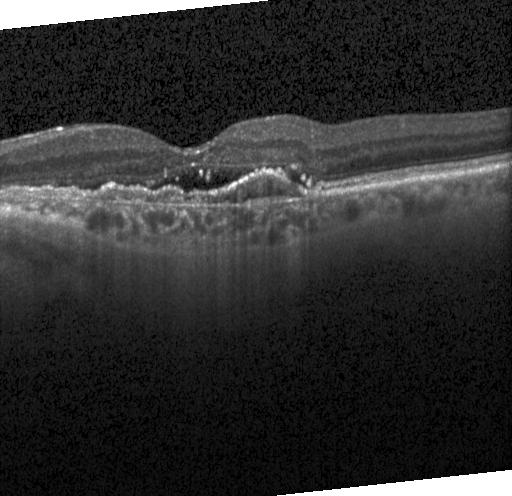
The scan shows choroidal neovascularization.